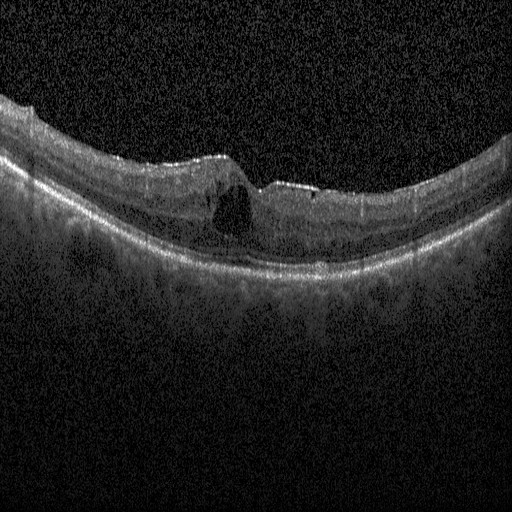 Macular OCT demonstrating DME.